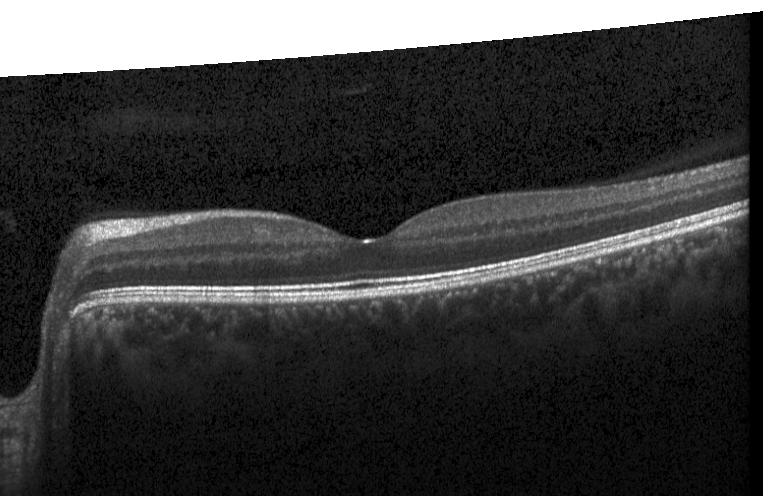

Spectral-domain OCT · fovea-centered · optical coherence tomography B-scan — Impression: no choroidal neovascularization, no diabetic macular edema, and no drusen.